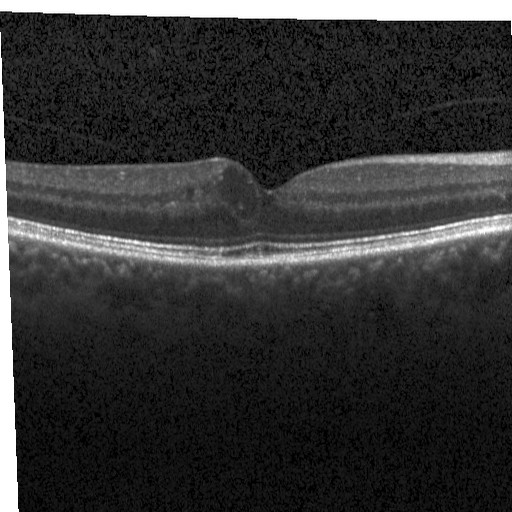

Optical coherence tomography B-scan; horizontal scan through the fovea; Heidelberg Spectralis
Assessment: diabetic macular edema.